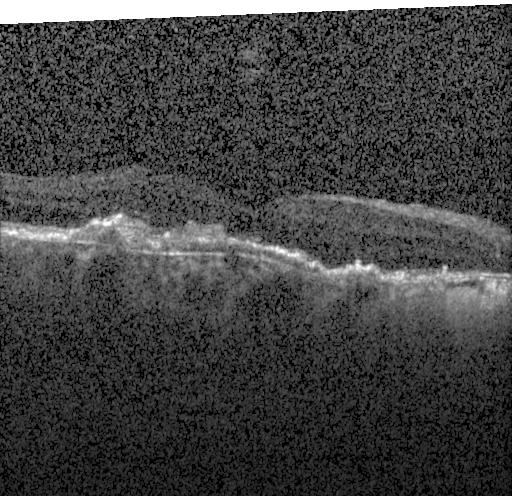
Diagnosis: choroidal neovascularization.